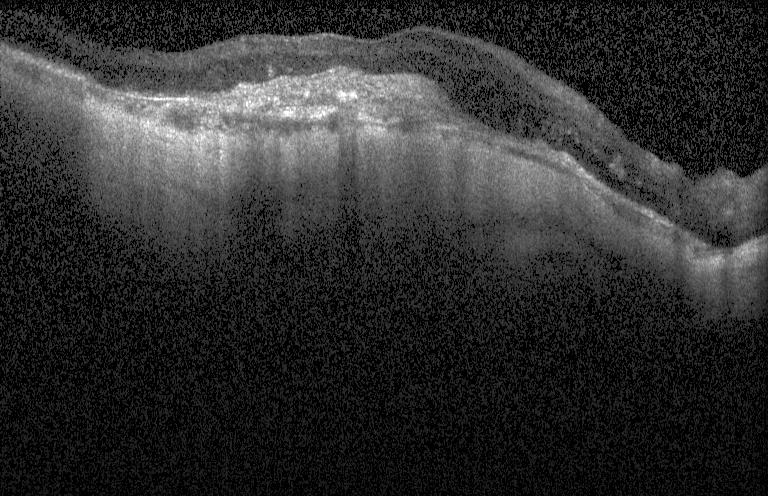
OCT B-scan; instrument: Heidelberg Spectralis.
Macular OCT: choroidal neovascularization.